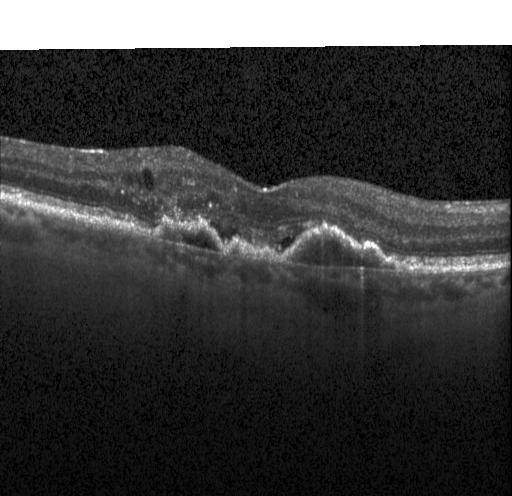

Diagnosis: a choroidal neovascular membrane.